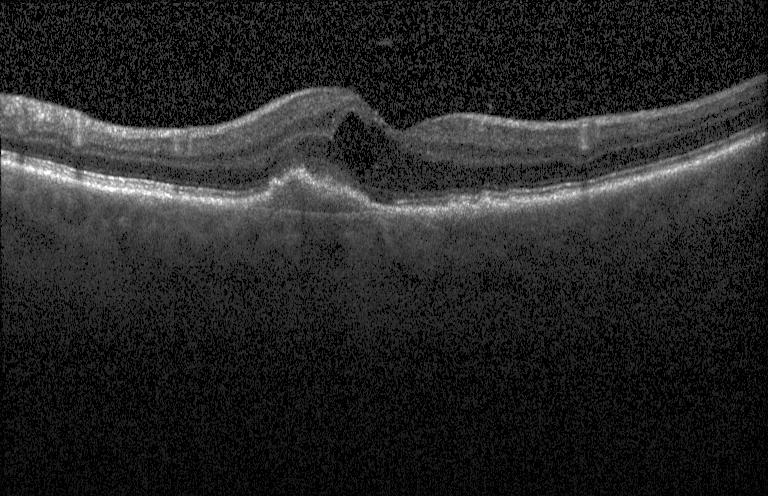
Instrument: Heidelberg Spectralis · SD-OCT · OCT line scan.
Assessment: a choroidal neovascular membrane.